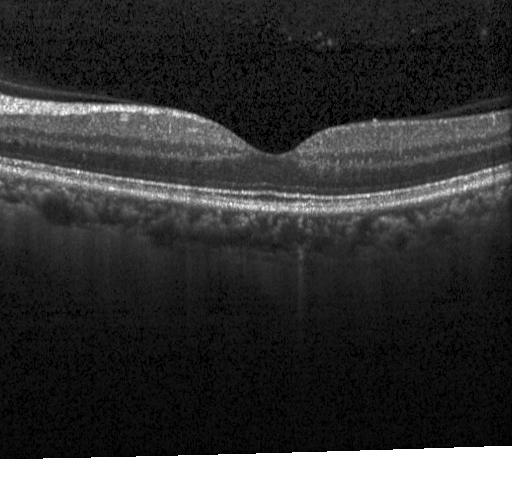
Horizontal scan through the fovea · retinal OCT cross-section — Finding: neither choroidal neovascularization, diabetic macular edema, nor drusen.